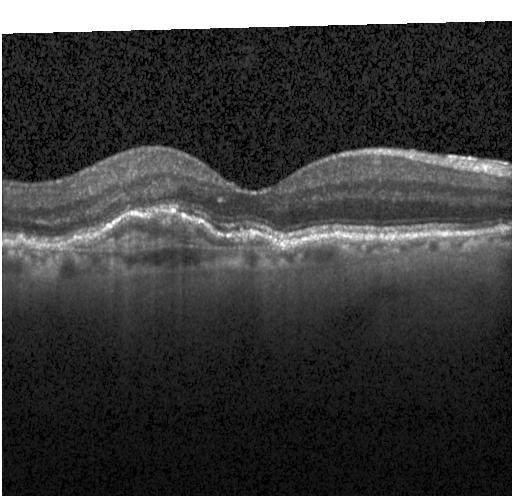

OCT line scan
The scan shows choroidal neovascularization.